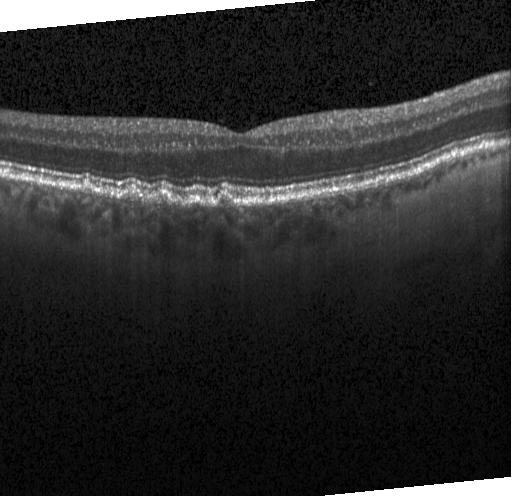
Heidelberg Spectralis OCT system. SD-OCT. OCT B-scan
Diagnosis: drusen.